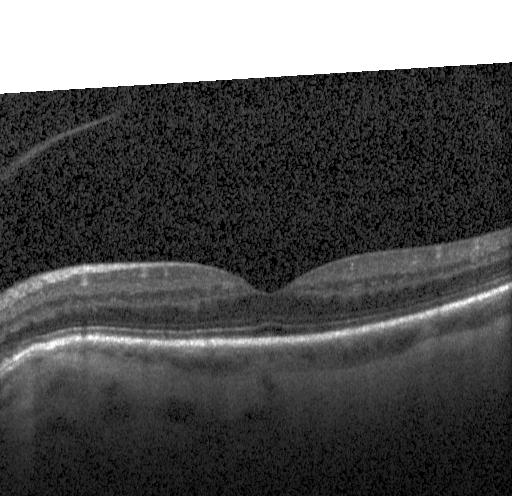

Finding: no choroidal neovascularization, no diabetic macular edema, and no drusen.